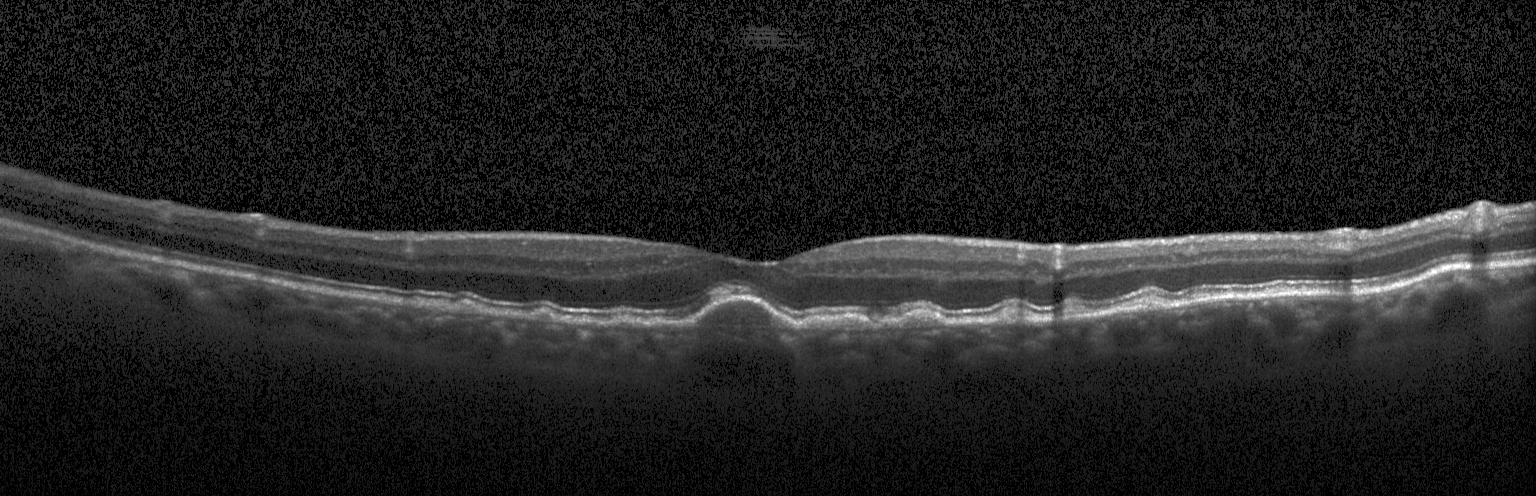

Heidelberg Spectralis · retinal OCT cross-section · SD-OCT.
Finding: drusen.